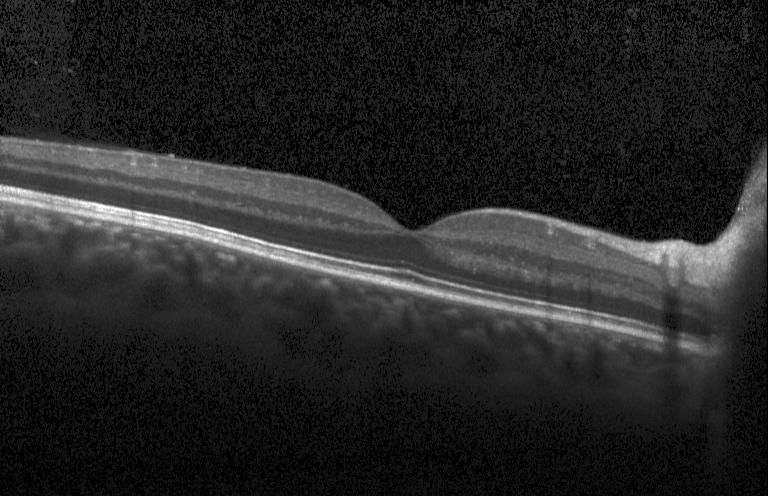 Diagnosis: neither CNV, DME, nor drusen.